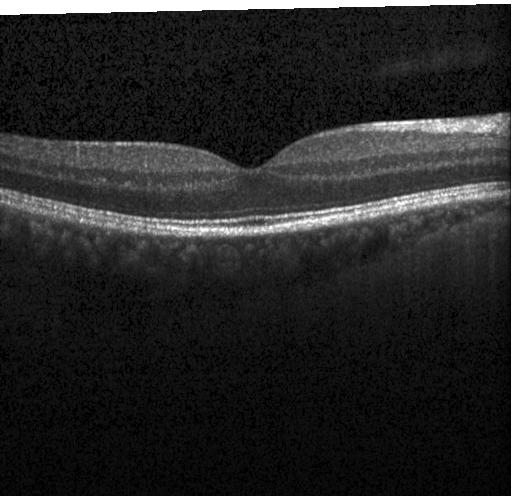

Optical coherence tomography scan; instrument: Heidelberg Spectralis — Impression: no evidence of CNV, DME, or drusen.